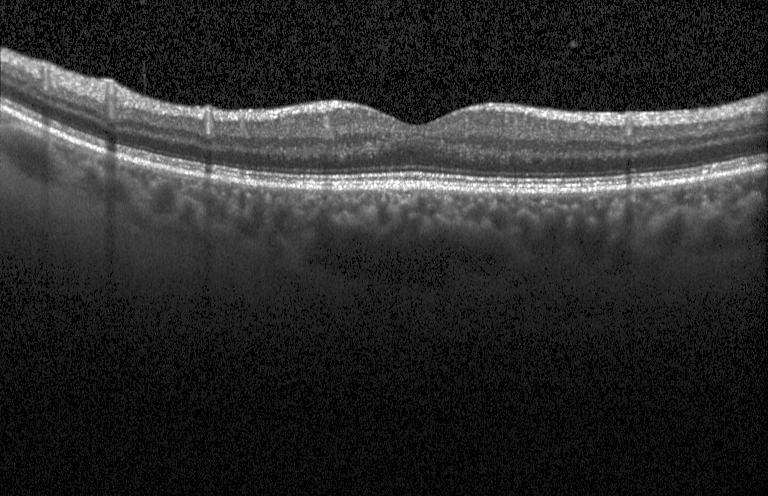
Retinal OCT B-scan.
Impression: no choroidal neovascularization, diabetic macular edema, or drusen.